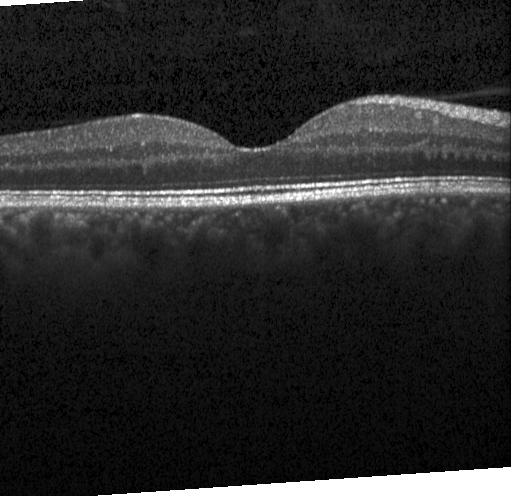
OCT line scan, acquired on a Heidelberg Spectralis, spectral-domain optical coherence tomography — Finding: no CNV, no DME, and no drusen.